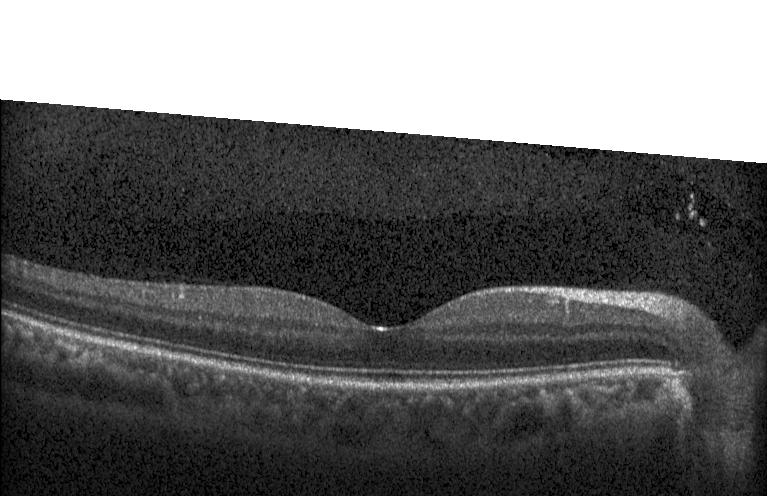

Finding: neither choroidal neovascularization, diabetic macular edema, nor drusen.